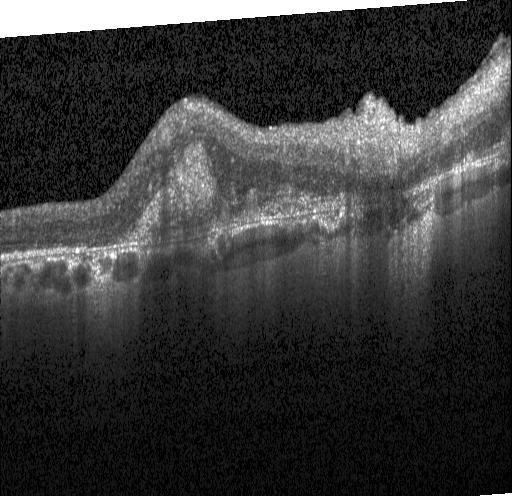

Retinal OCT B-scan, acquired on a Heidelberg Spectralis
Finding: a choroidal neovascular membrane.